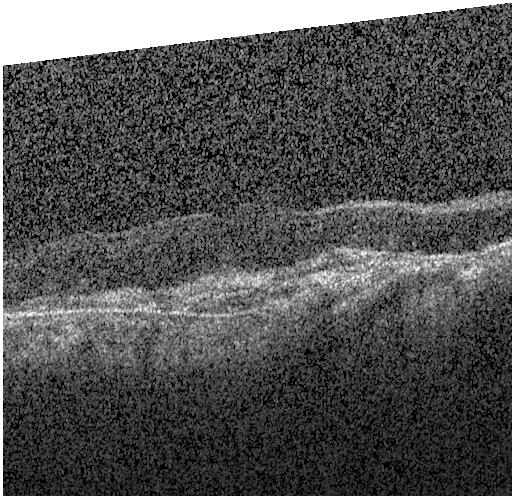
Acquired on a Heidelberg Spectralis; macular scan; spectral-domain optical coherence tomography; OCT line scan
Impression: CNV.